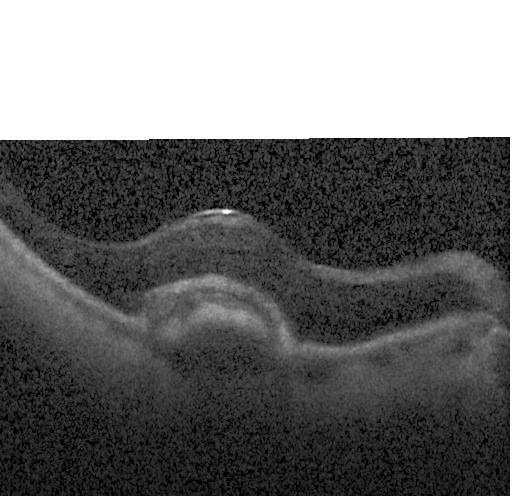 OCT line scan — Impression: choroidal neovascularization (CNV).